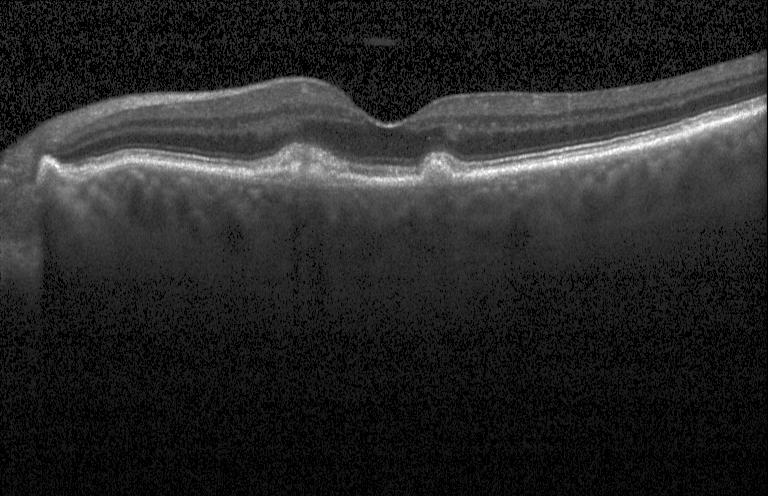 Spectral-domain OCT, Heidelberg Spectralis OCT system, retinal OCT B-scan.
Macular OCT: a choroidal neovascular membrane.